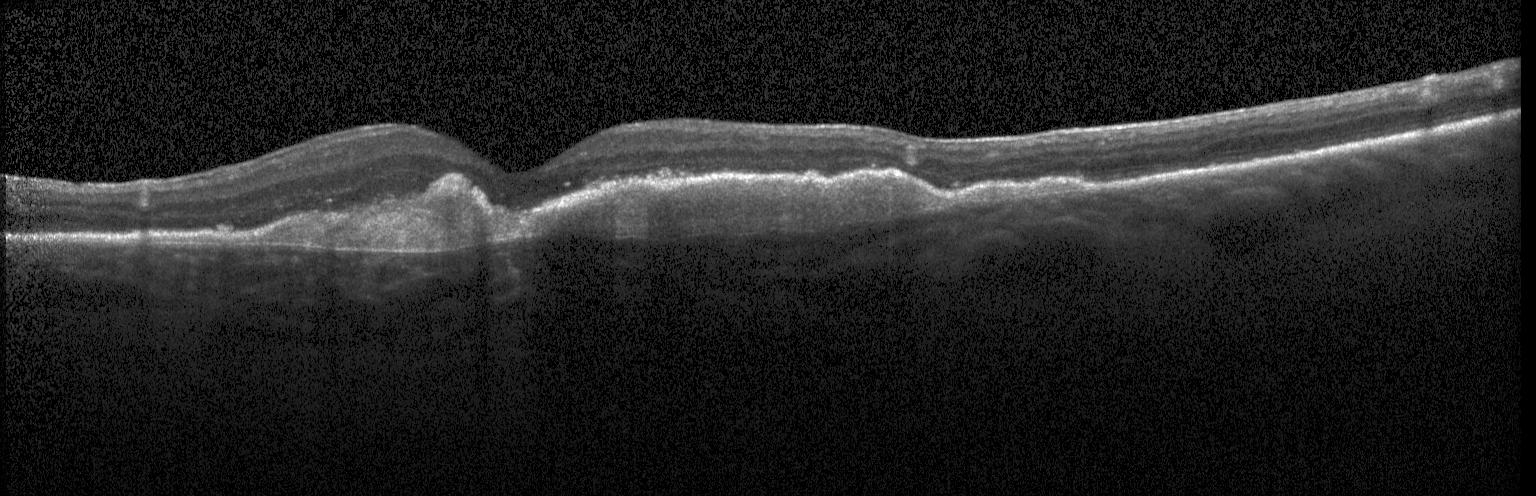
SD-OCT, OCT line scan, instrument: Heidelberg Spectralis, macular scan.
This B-scan demonstrates CNV.